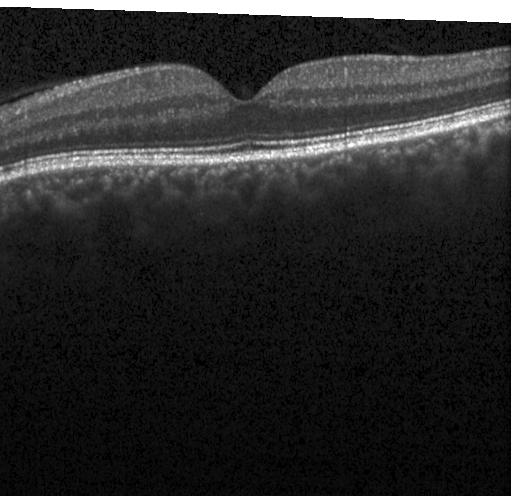 Macular OCT: no evidence of choroidal neovascularization, diabetic macular edema, or drusen.